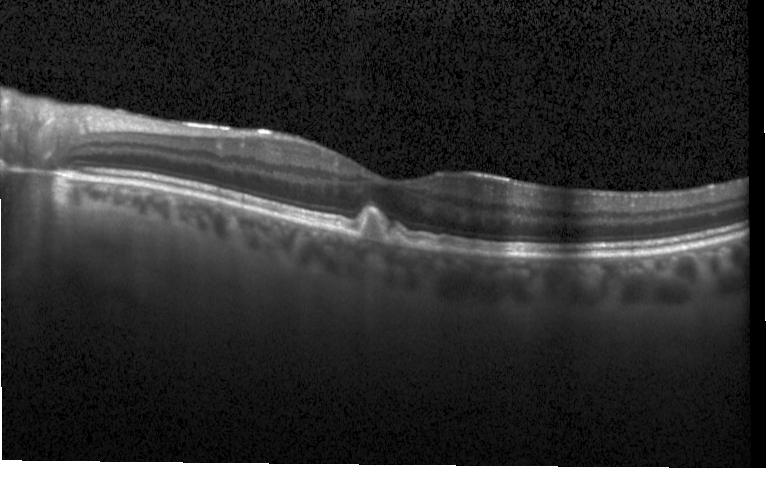

Dx: multiple drusen.